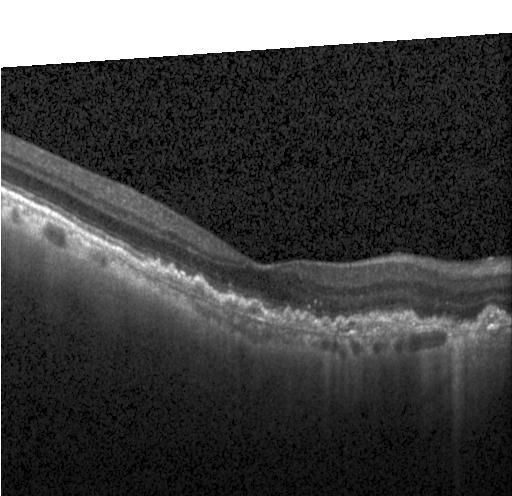

Optical coherence tomography B-scan, through the macula. Assessment: a choroidal neovascular membrane.